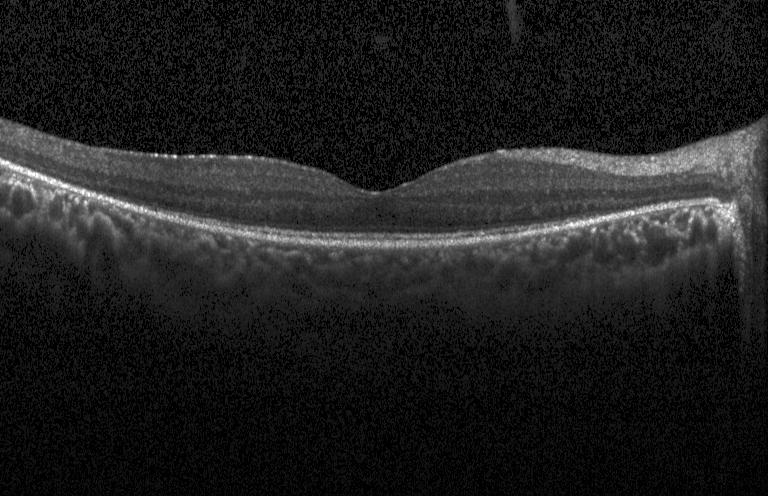
No CNV, no DME, and no drusen.